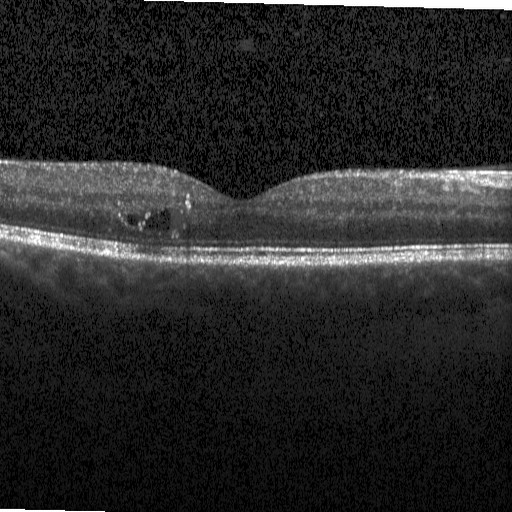 Acquired on a Heidelberg Spectralis. Optical coherence tomography scan
Diagnosis: diabetic macular edema (DME).